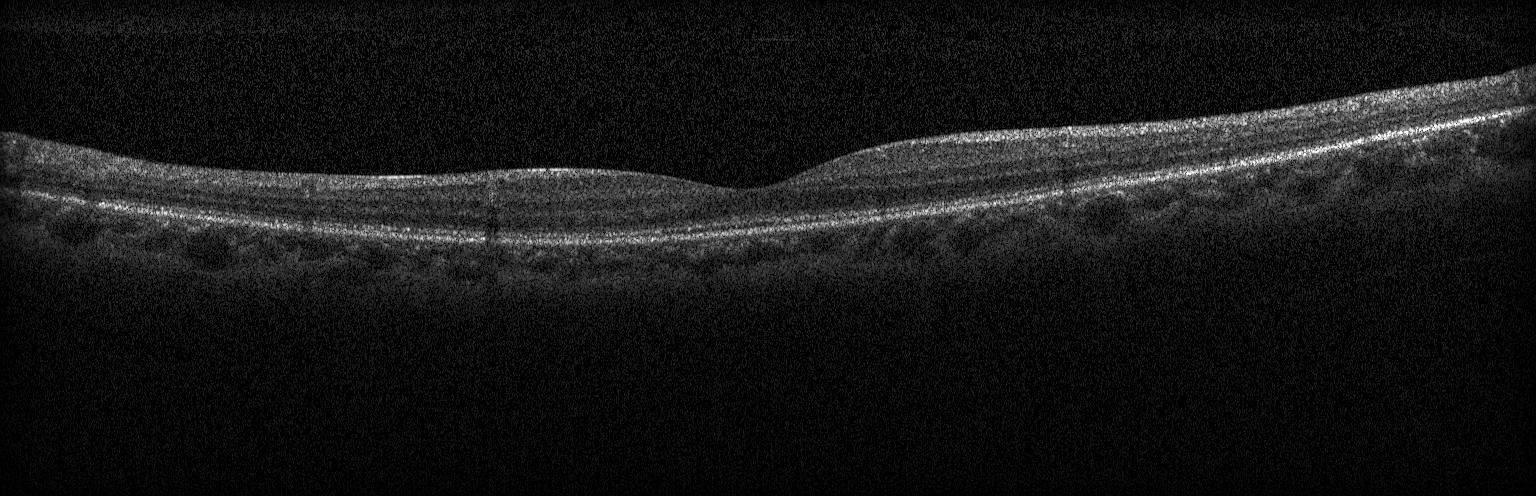
Dx: neither CNV, DME, nor drusen.